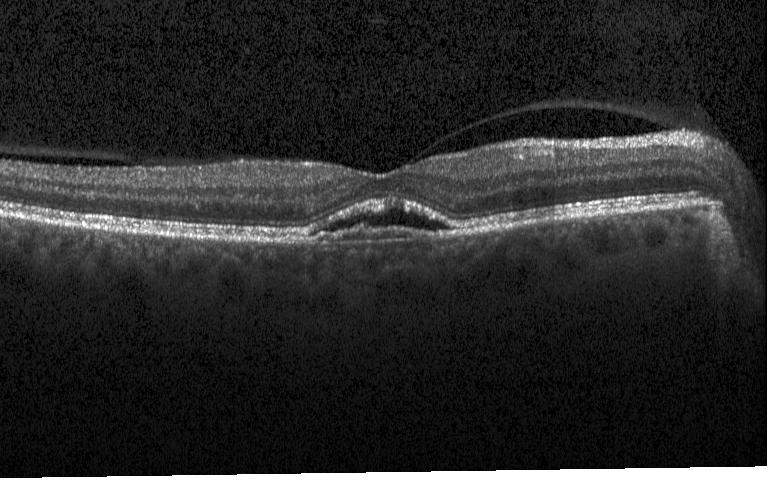
Impression: a choroidal neovascular membrane.